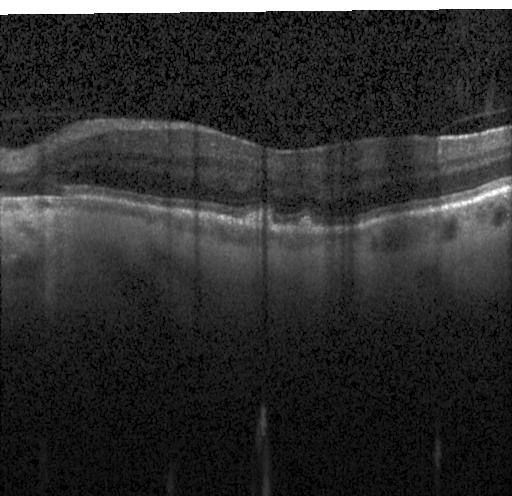
Assessment: multiple drusen.